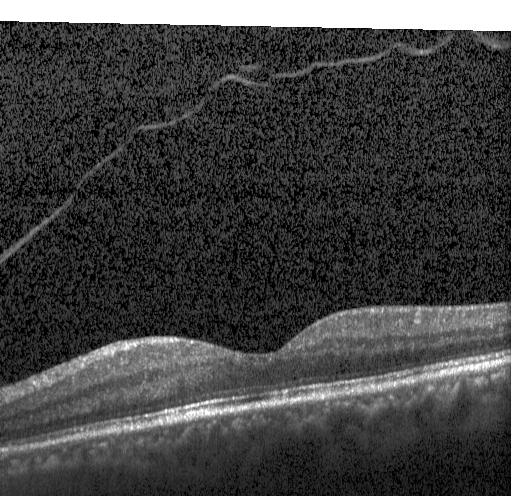
Horizontal scan through the fovea; optical coherence tomography scan; SD-OCT; Heidelberg Spectralis OCT system.
OCT finding: neither choroidal neovascularization, diabetic macular edema, nor drusen.